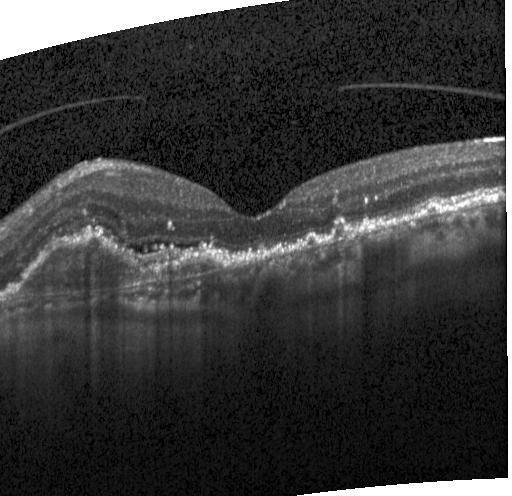 Heidelberg Spectralis OCT system; optical coherence tomography scan; horizontal scan through the fovea — A choroidal neovascular membrane.